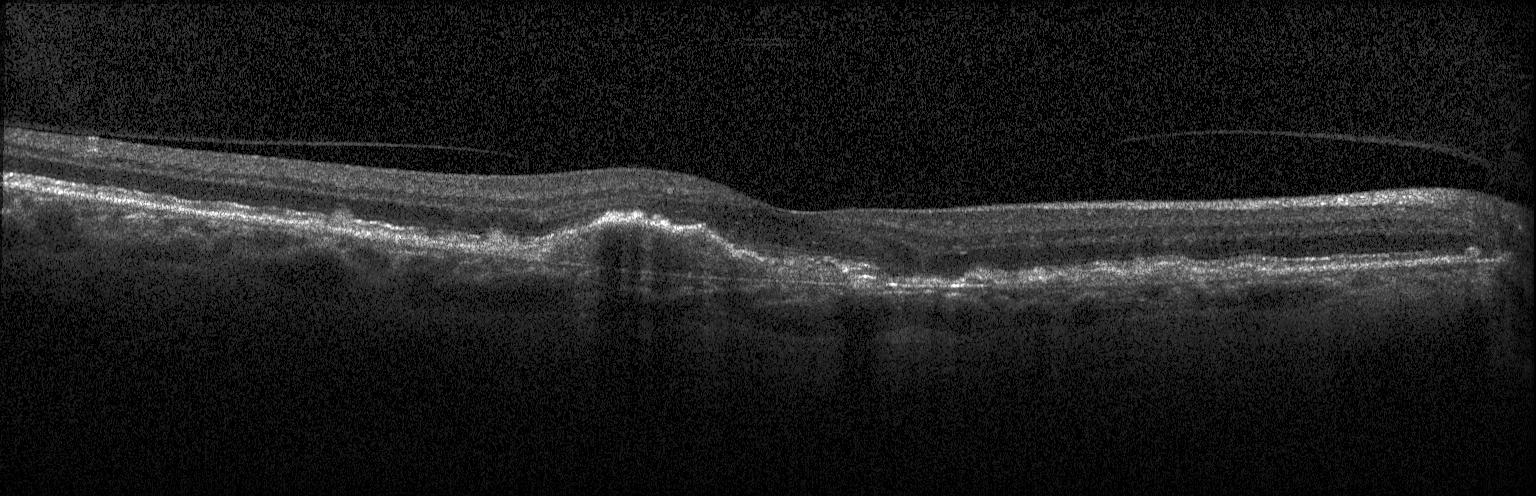

Macular OCT demonstrating choroidal neovascularization.